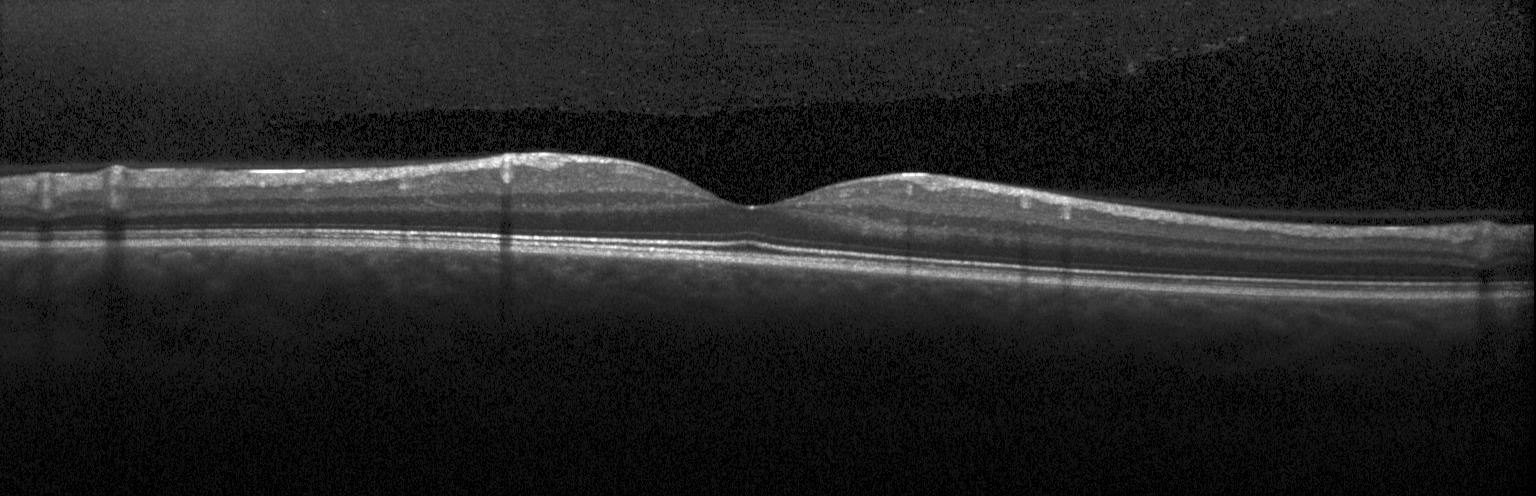

Acquired on a Heidelberg Spectralis · spectral-domain optical coherence tomography · optical coherence tomography scan
This B-scan demonstrates no choroidal neovascularization, diabetic macular edema, or drusen.